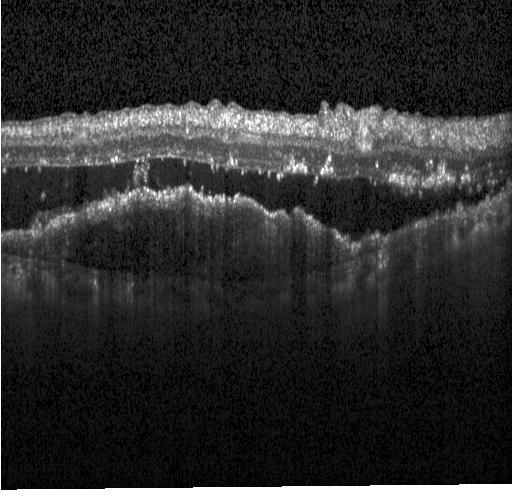 This B-scan demonstrates a choroidal neovascular membrane.